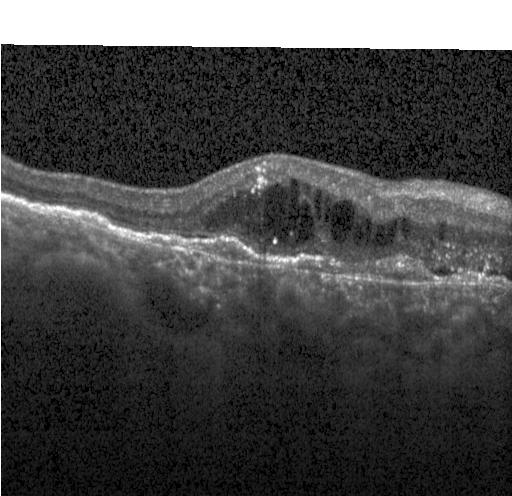

Diagnosis: choroidal neovascularization (CNV).